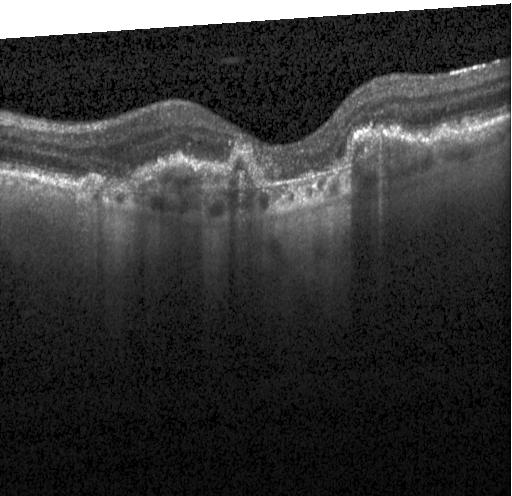
Spectral-domain OCT B-scan: choroidal neovascularization.